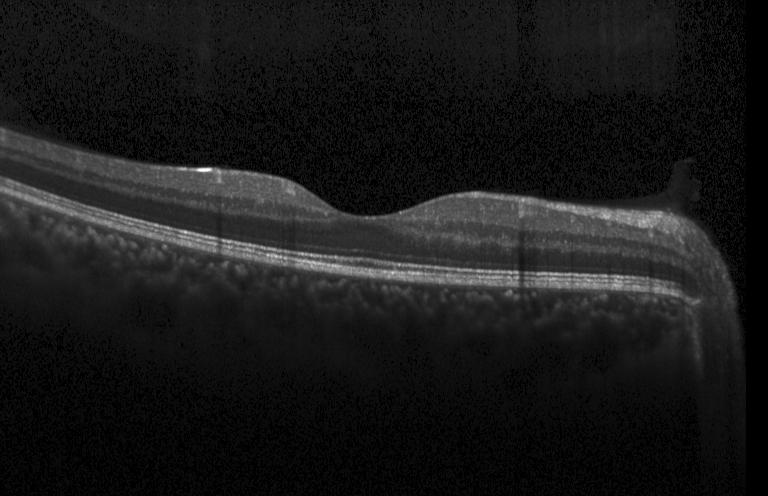
Spectral-domain OCT; instrument: Heidelberg Spectralis; centered on the fovea; optical coherence tomography scan. Assessment: no evidence of choroidal neovascularization, diabetic macular edema, or drusen.